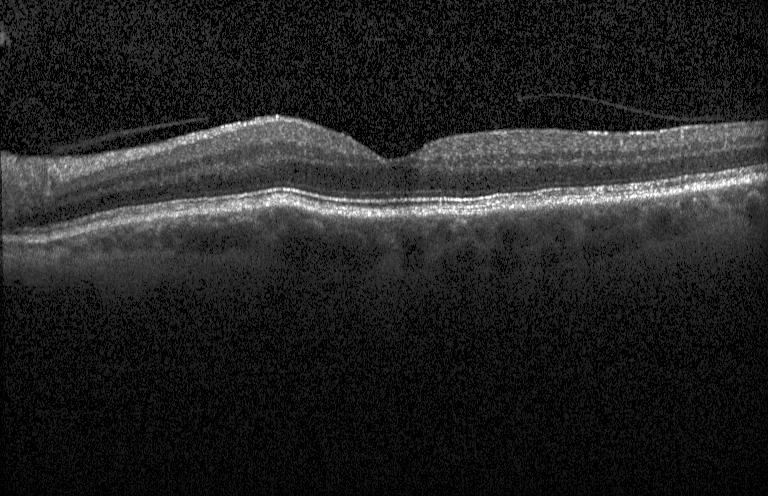 Horizontal scan through the fovea · OCT line scan. Impression: neither choroidal neovascularization, diabetic macular edema, nor drusen.